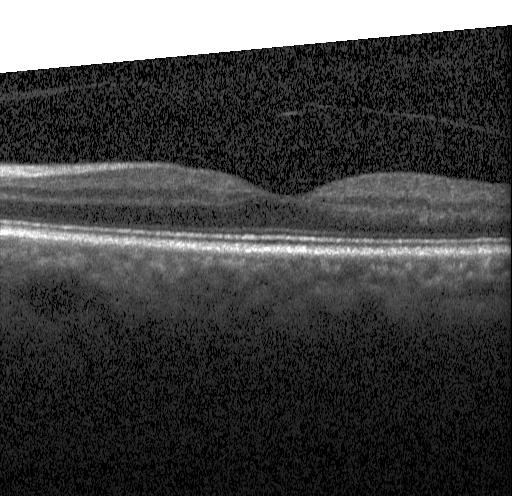

Retinal OCT cross-section; SD-OCT. Macular OCT: neither choroidal neovascularization, diabetic macular edema, nor drusen.